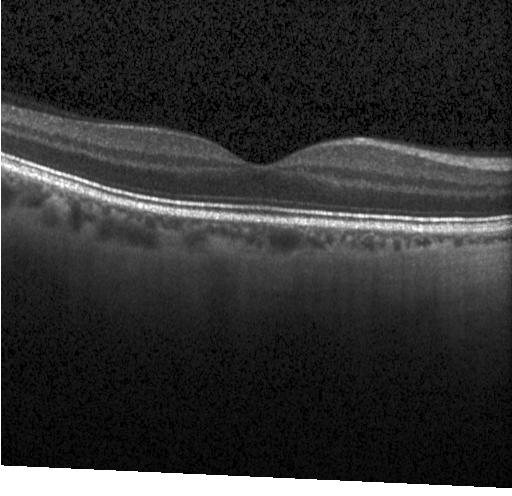

Assessment: no CNV, DME, or drusen.